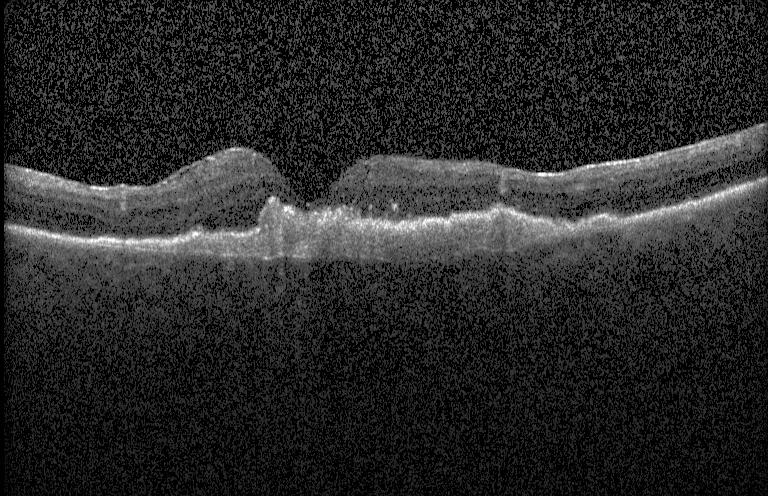

Optical coherence tomography B-scan — The scan shows CNV.